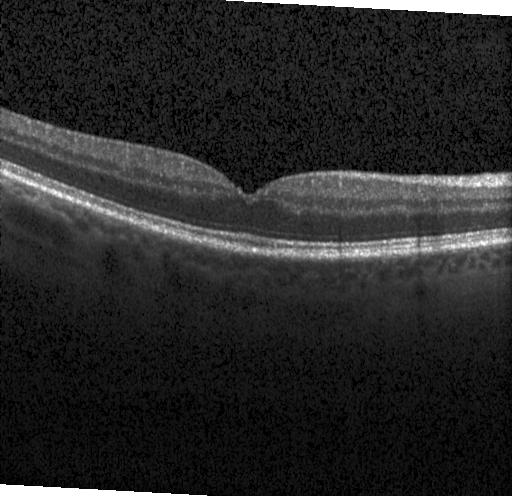 Optical coherence tomography B-scan, macular scan — Finding: no CNV, DME, or drusen.